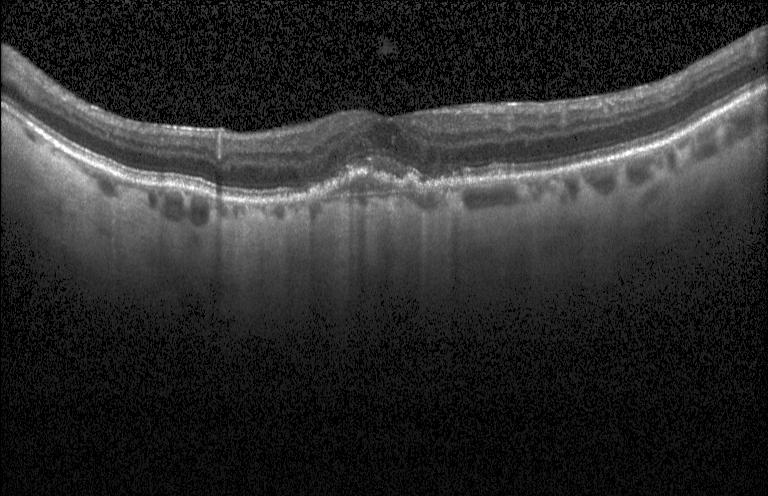
A choroidal neovascular membrane.